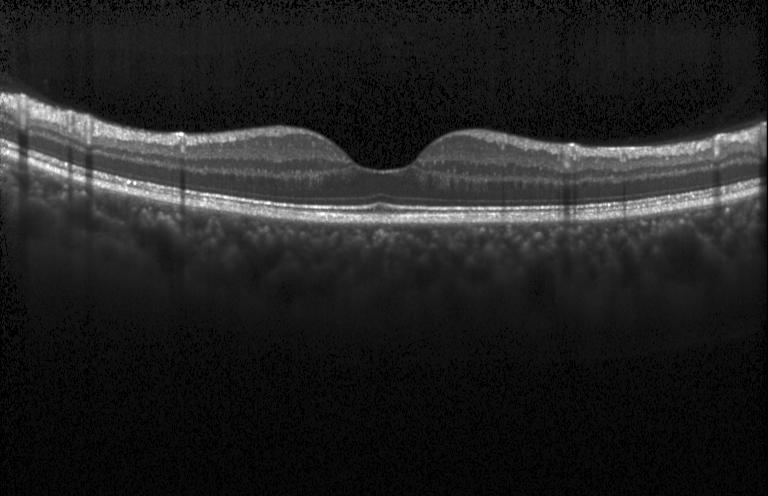

Through the macula · Heidelberg Spectralis · SD-OCT · retinal OCT B-scan.
Impression: no choroidal neovascularization, no diabetic macular edema, and no drusen.